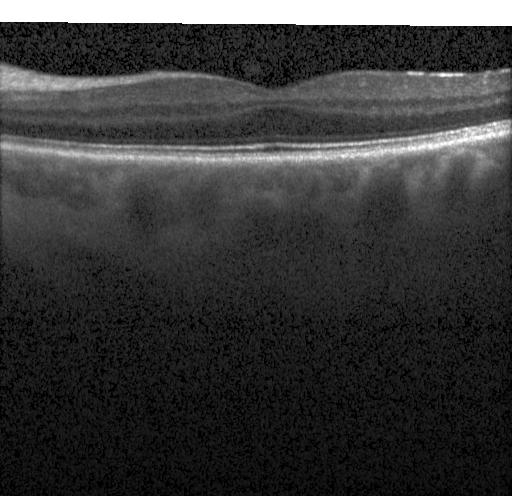
Assessment: neither choroidal neovascularization, diabetic macular edema, nor drusen.